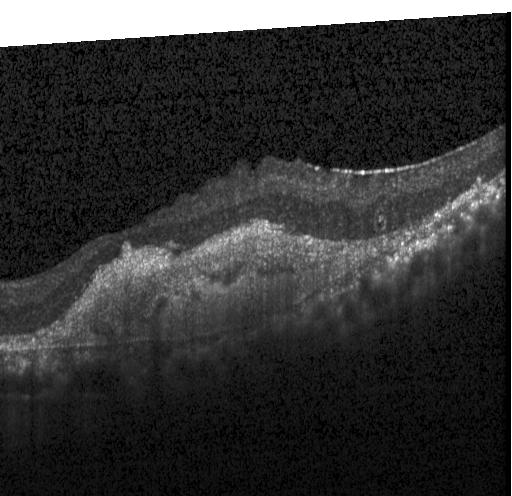

Optical coherence tomography B-scan.
Diagnosis: CNV.